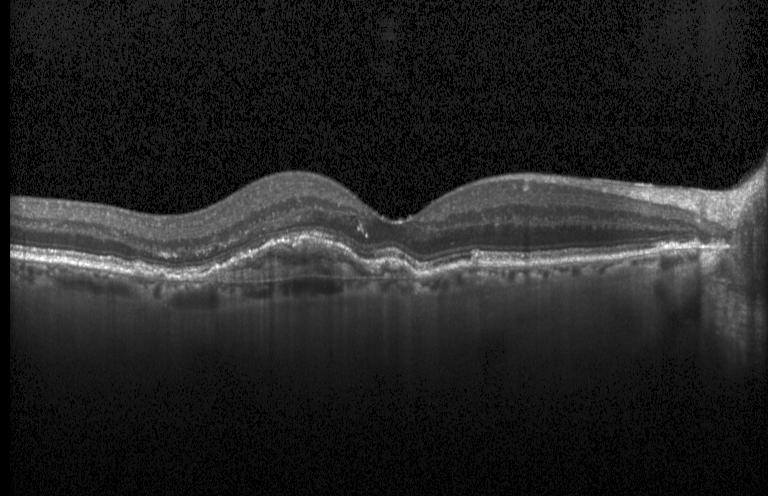 Optical coherence tomography scan · instrument: Heidelberg Spectralis. Dx: a choroidal neovascular membrane.